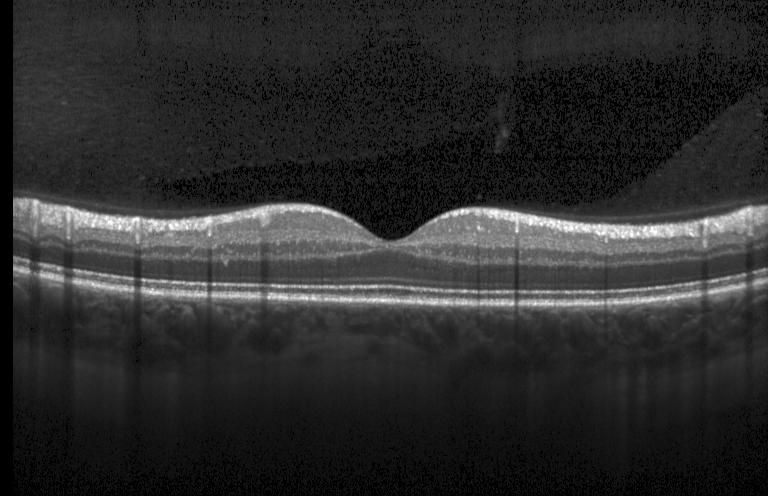 Retinal OCT cross-section; through the macula — Assessment: no CNV, no DME, and no drusen.